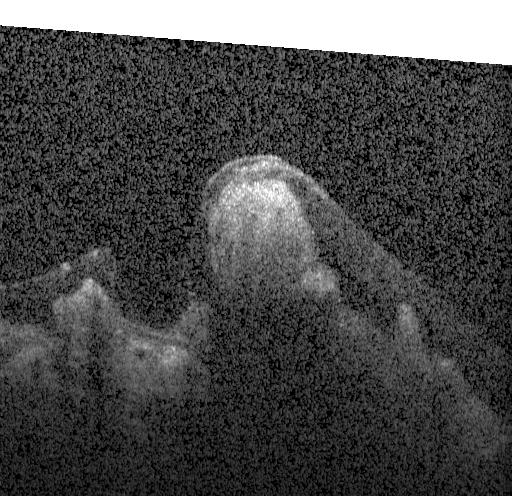 OCT B-scan, spectral-domain optical coherence tomography. This B-scan demonstrates CNV.